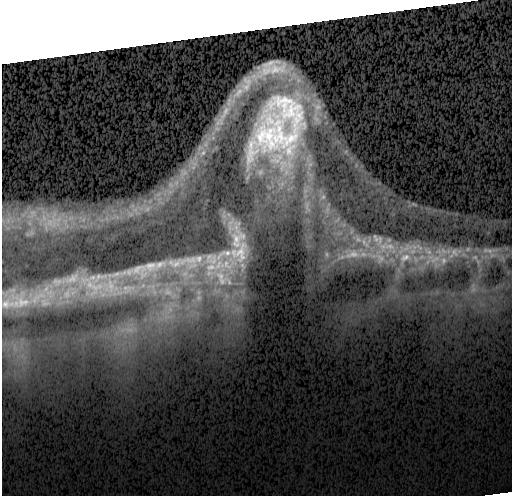

Dx: choroidal neovascularization.